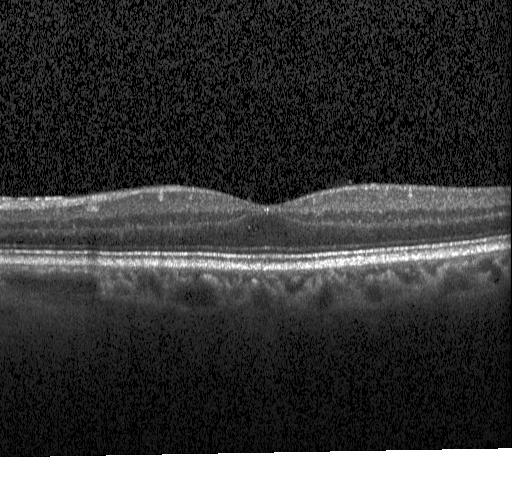

Heidelberg Spectralis; spectral-domain optical coherence tomography; retinal OCT B-scan; centered on the fovea. This B-scan demonstrates no choroidal neovascularization, diabetic macular edema, or drusen.